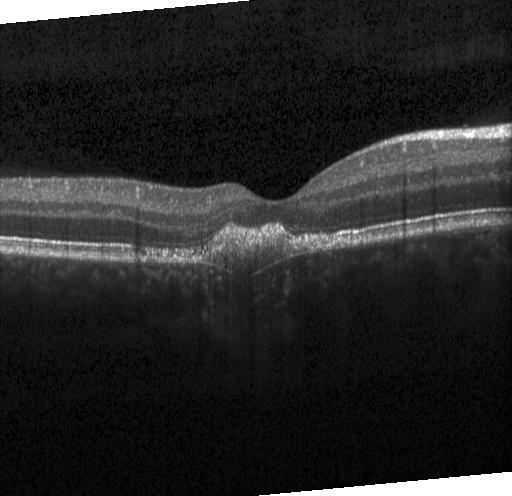
Retinal OCT B-scan — Impression: CNV.